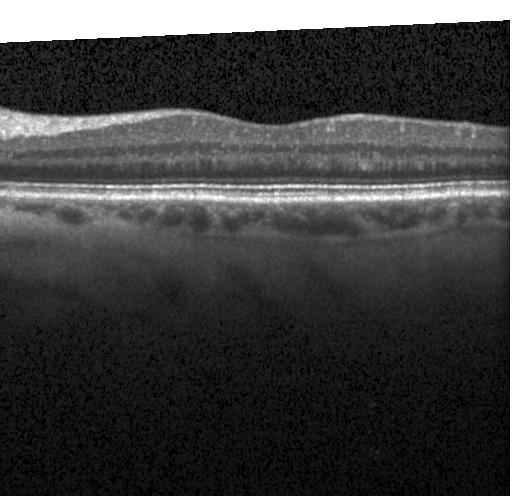

Spectral-domain OCT. Horizontal scan through the fovea. OCT B-scan — Assessment: no choroidal neovascularization, diabetic macular edema, or drusen.